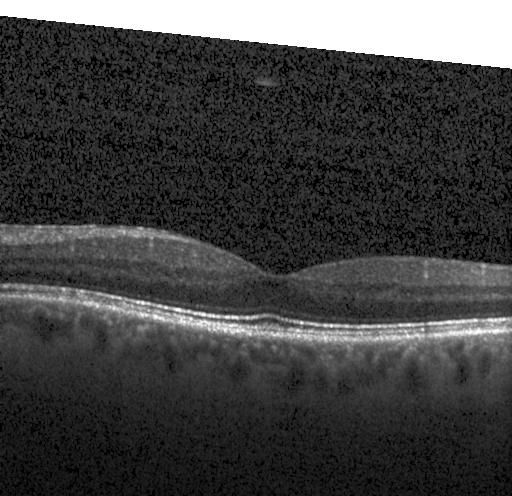
Spectral-domain optical coherence tomography · retinal OCT cross-section · centered on the fovea · Heidelberg Spectralis — Diagnosis: no evidence of choroidal neovascularization, diabetic macular edema, or drusen.